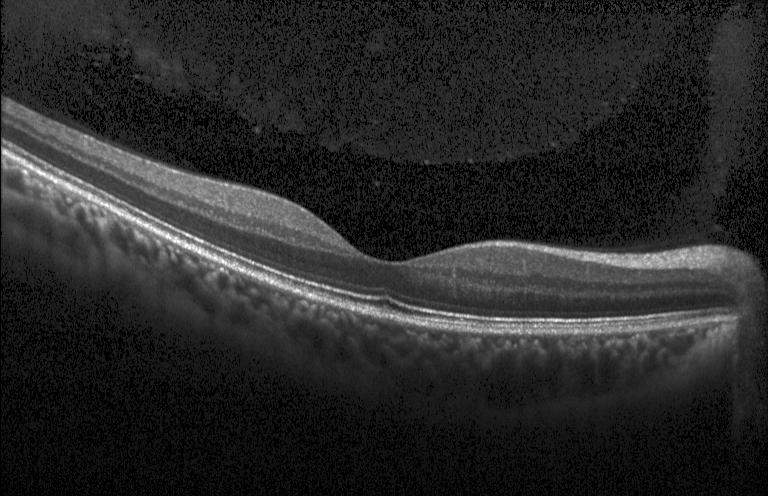 OCT B-scan showing no evidence of choroidal neovascularization, diabetic macular edema, or drusen.